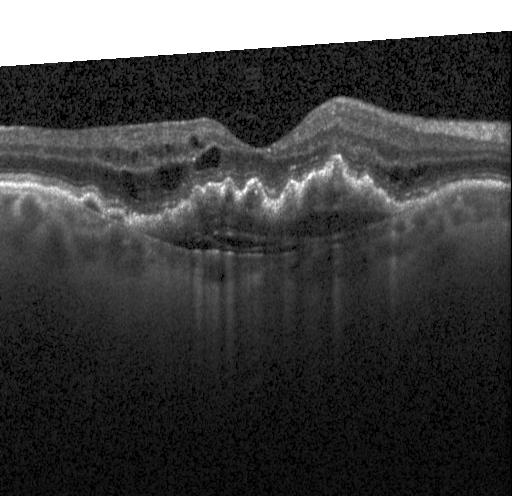
OCT line scan · acquired on a Heidelberg Spectralis.
Macular OCT: a choroidal neovascular membrane.